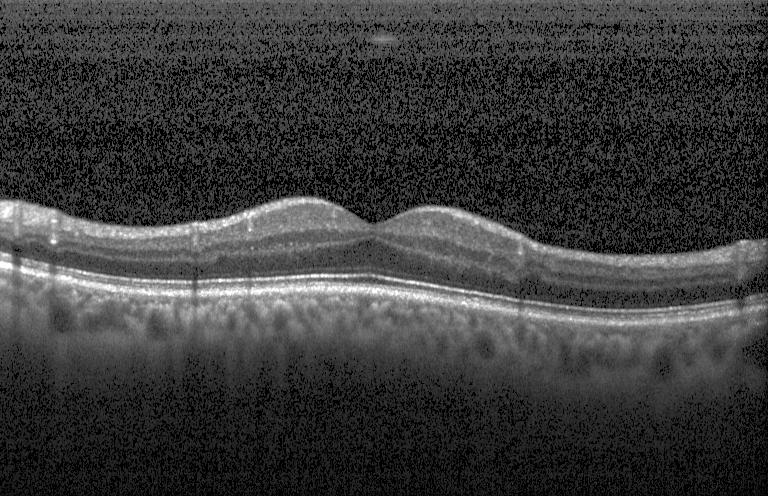
Impression: no CNV, DME, or drusen.